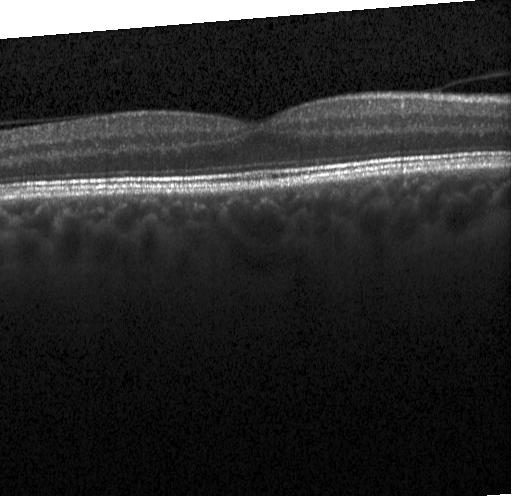

Spectral-domain OCT, retinal OCT B-scan, through the macula, Heidelberg Spectralis.
Finding: no evidence of choroidal neovascularization, diabetic macular edema, or drusen.